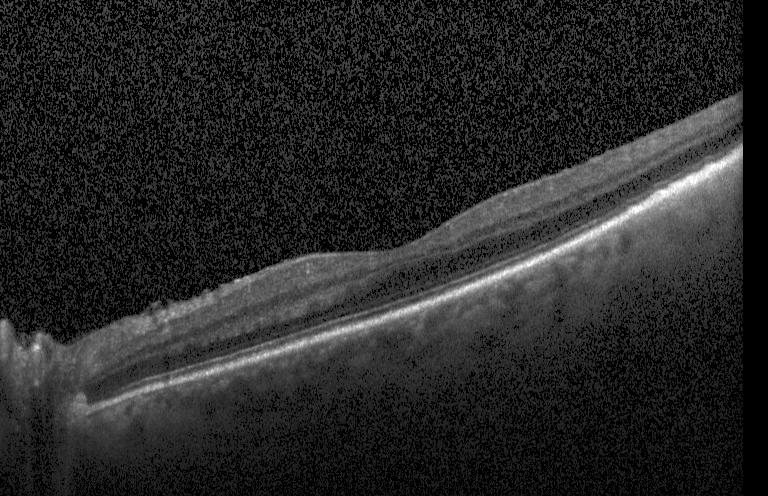 Impression: no choroidal neovascularization, no diabetic macular edema, and no drusen.